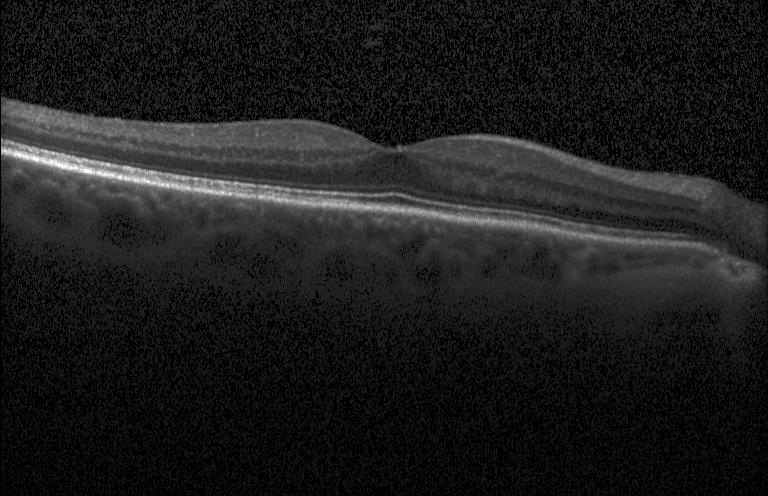 OCT finding: no evidence of choroidal neovascularization, diabetic macular edema, or drusen.